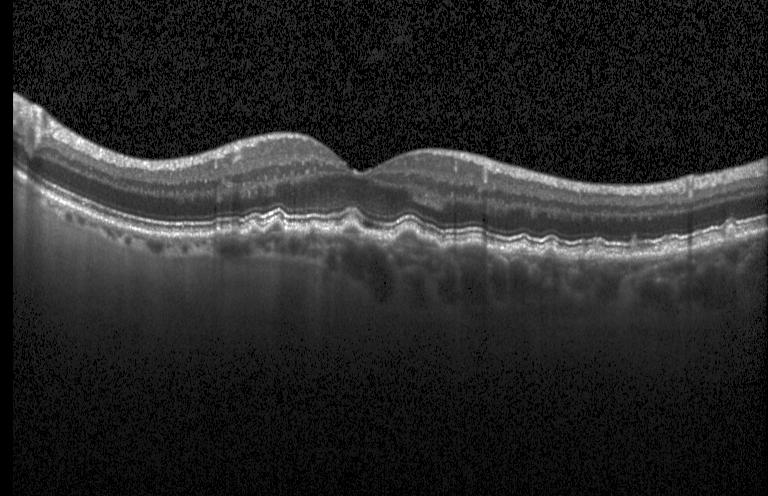 SD-OCT. Acquired on a Heidelberg Spectralis. Retinal OCT cross-section. Through the macula
Finding: multiple drusen.